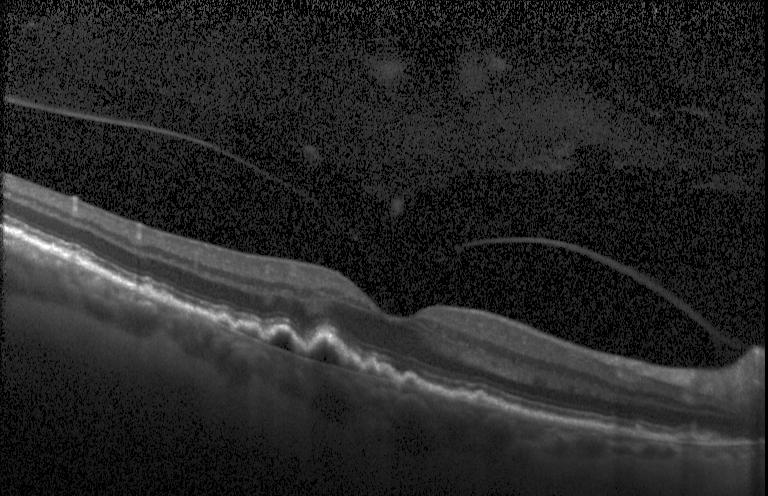

Acquired on a Heidelberg Spectralis. Retinal OCT B-scan
A choroidal neovascular membrane.